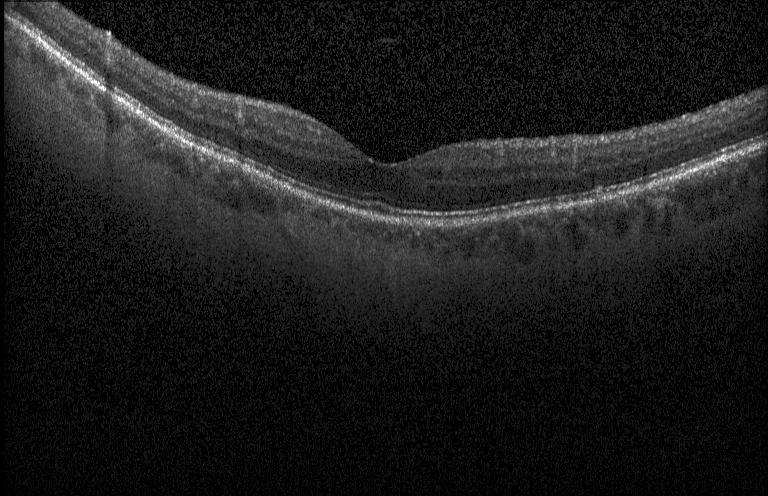 Macular scan, Heidelberg Spectralis OCT system, OCT line scan
OCT finding: neither choroidal neovascularization, diabetic macular edema, nor drusen.